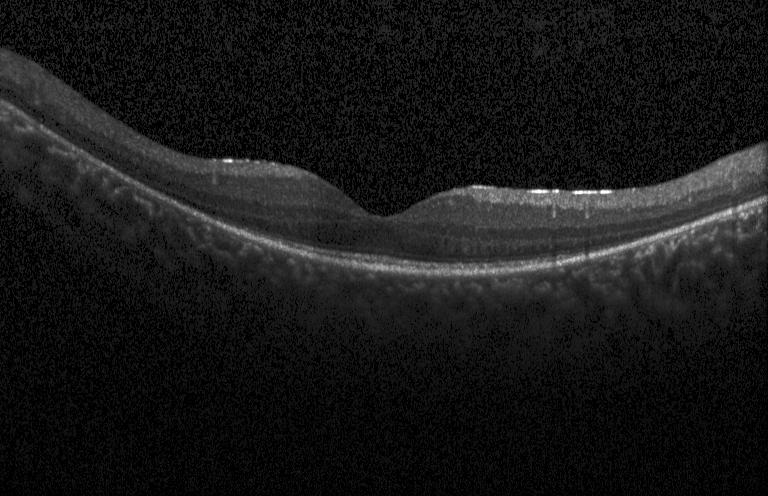 Diagnosis: no evidence of choroidal neovascularization, diabetic macular edema, or drusen.